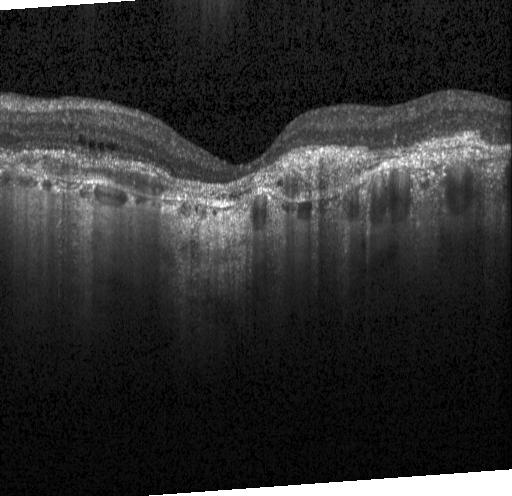
OCT B-scan.
Impression: a choroidal neovascular membrane.